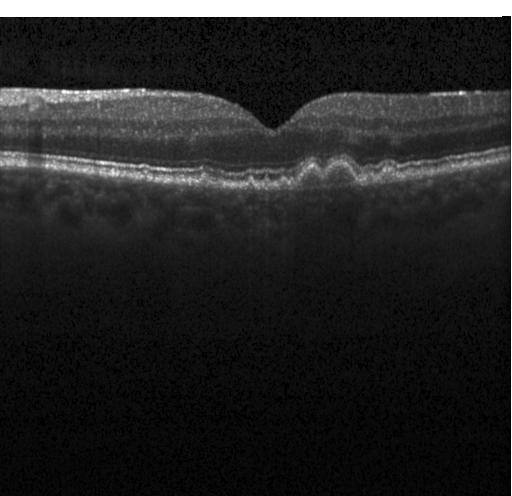 OCT B-scan showing sub-RPE drusenoid deposits.